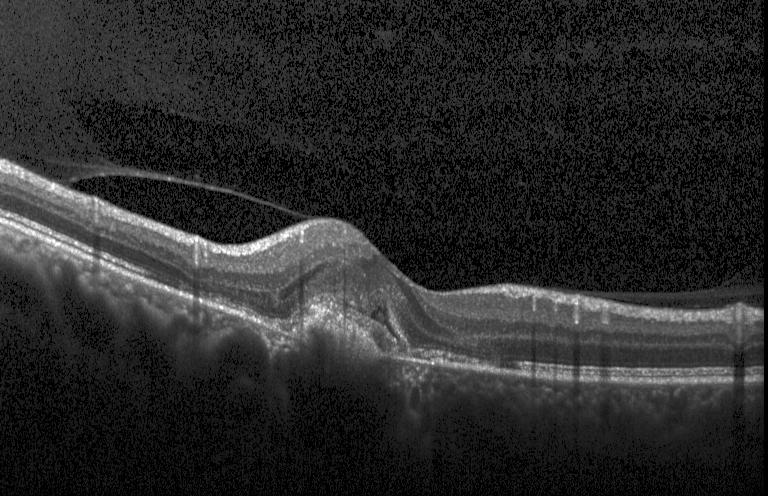
Instrument: Heidelberg Spectralis; retinal OCT cross-section
Finding: CNV.